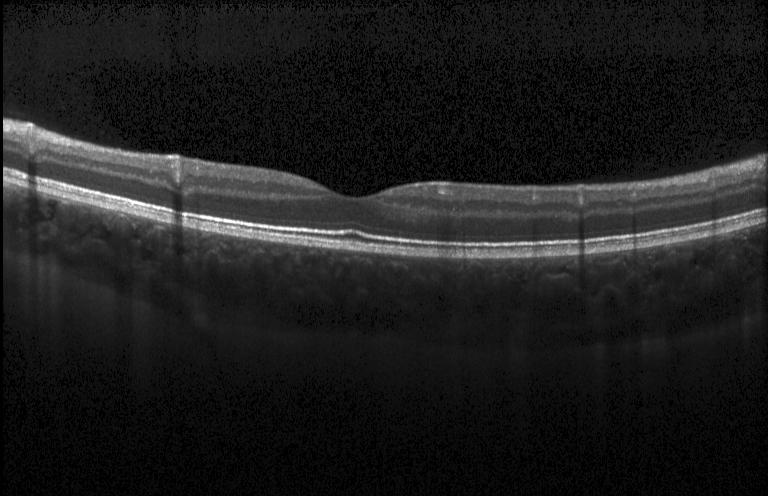

Centered on the fovea; spectral-domain OCT; OCT B-scan; instrument: Heidelberg Spectralis.
Dx: neither choroidal neovascularization, diabetic macular edema, nor drusen.